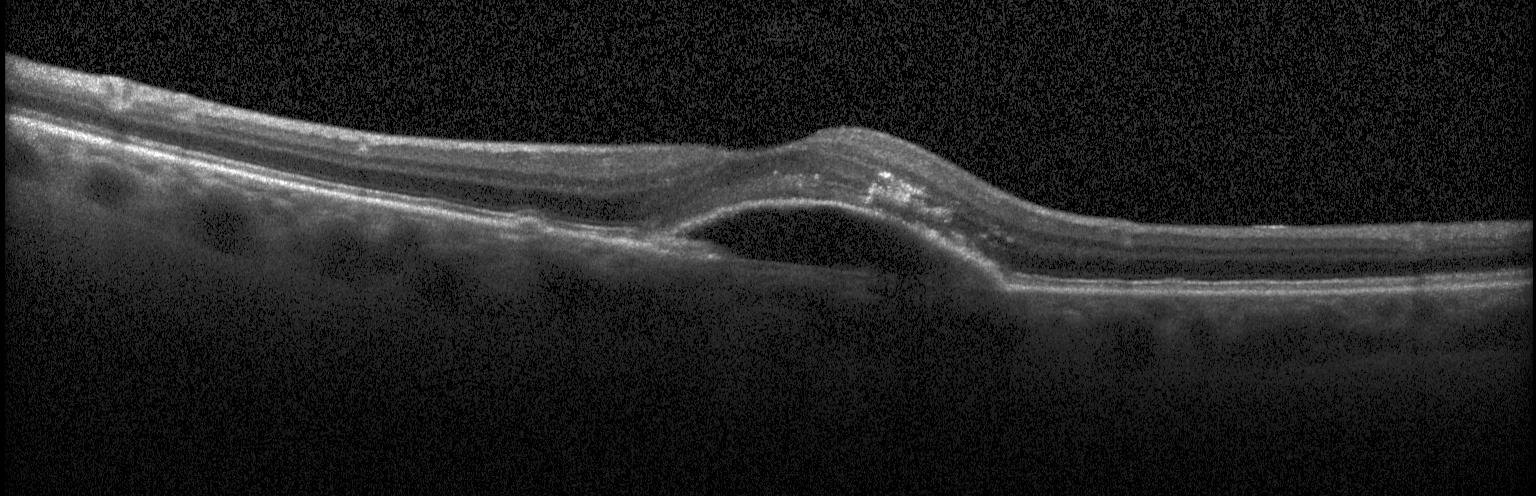

This B-scan demonstrates CNV.